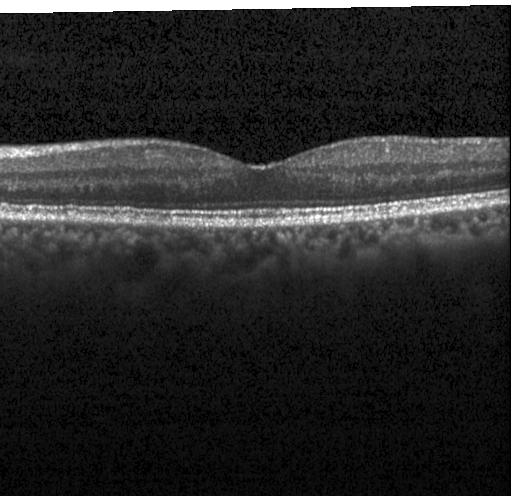 Impression: no evidence of choroidal neovascularization, diabetic macular edema, or drusen.